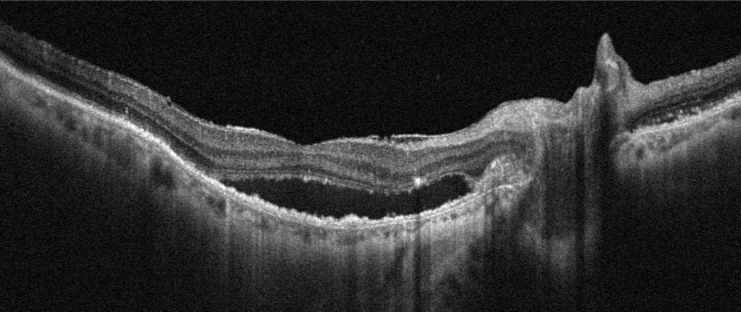
Retinal OCT cross-section showing AMD.